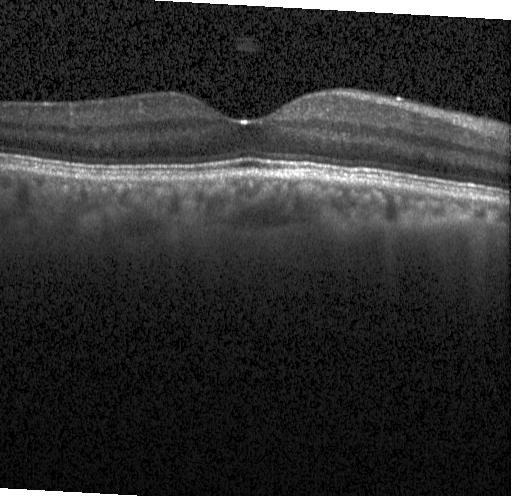 Impression: no CNV, DME, or drusen.